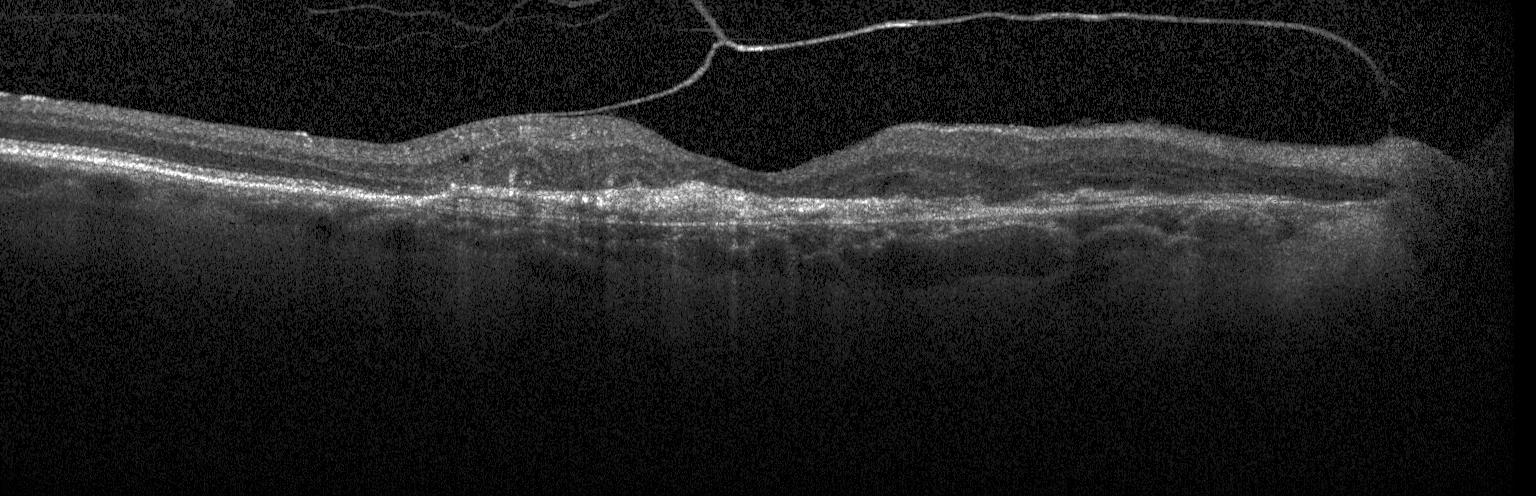
Spectral-domain OCT B-scan: choroidal neovascularization (CNV).